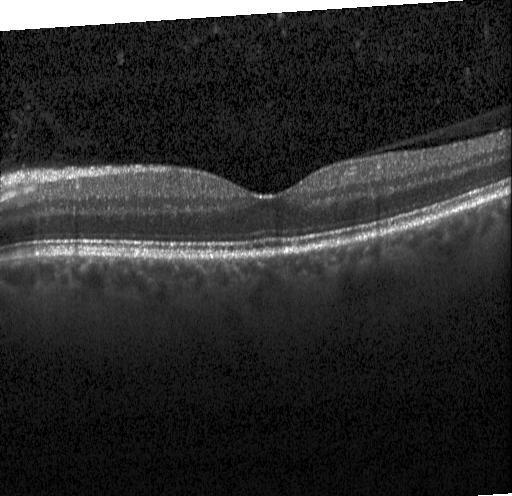
The scan shows no CNV, DME, or drusen.